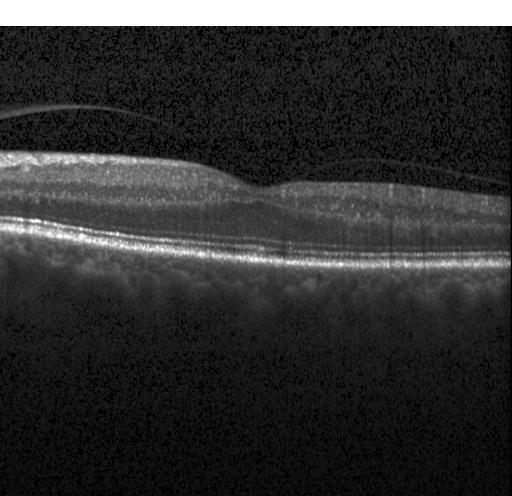
Finding: no CNV, no DME, and no drusen.